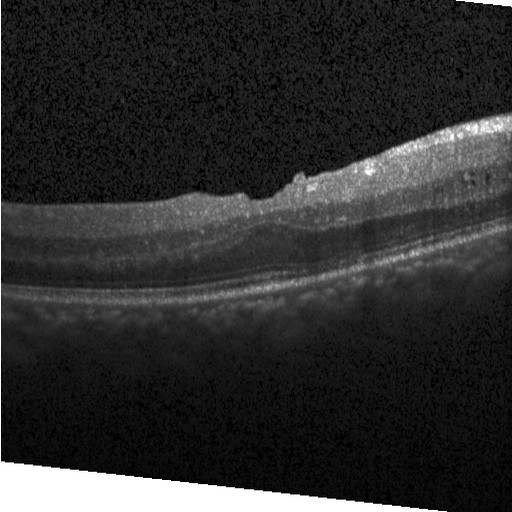

Heidelberg Spectralis OCT system. OCT line scan
This B-scan demonstrates diabetic macular edema.